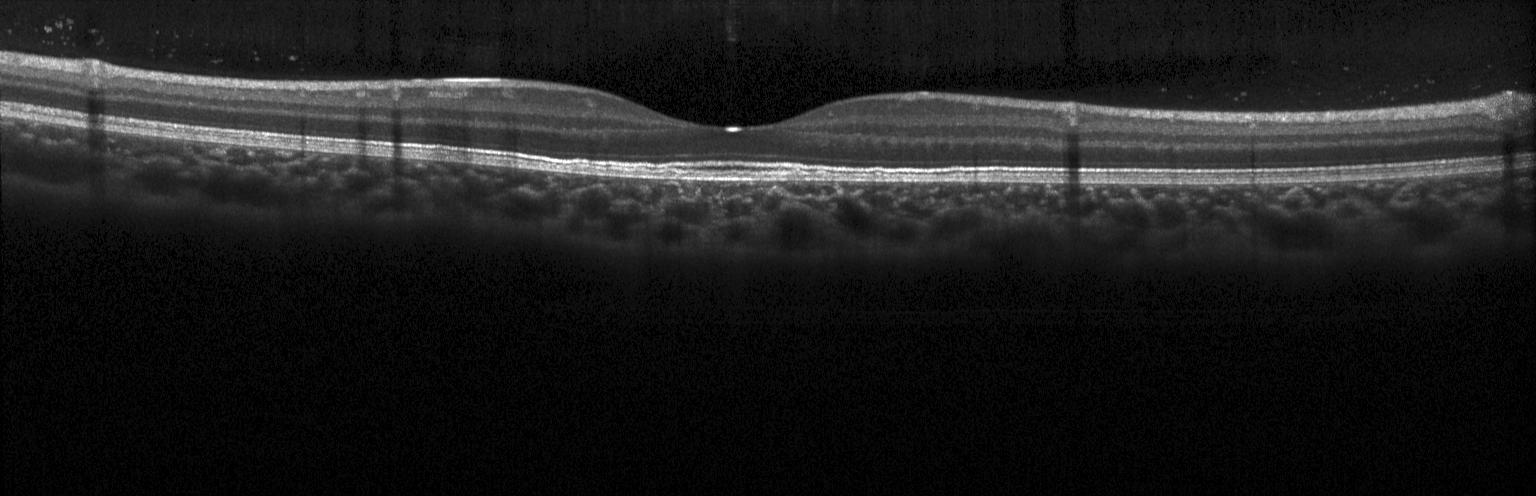

Dx: no evidence of choroidal neovascularization, diabetic macular edema, or drusen.